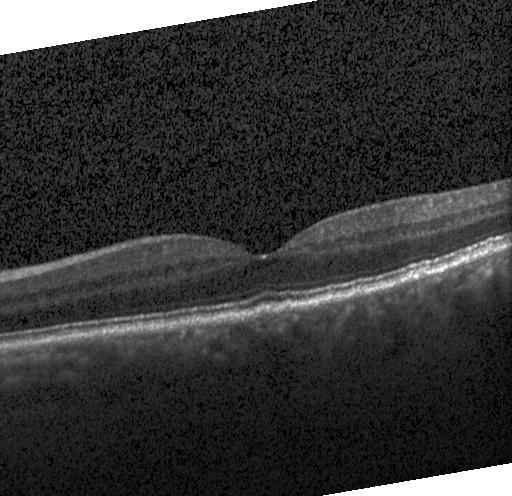 Macular OCT demonstrating multiple drusen.